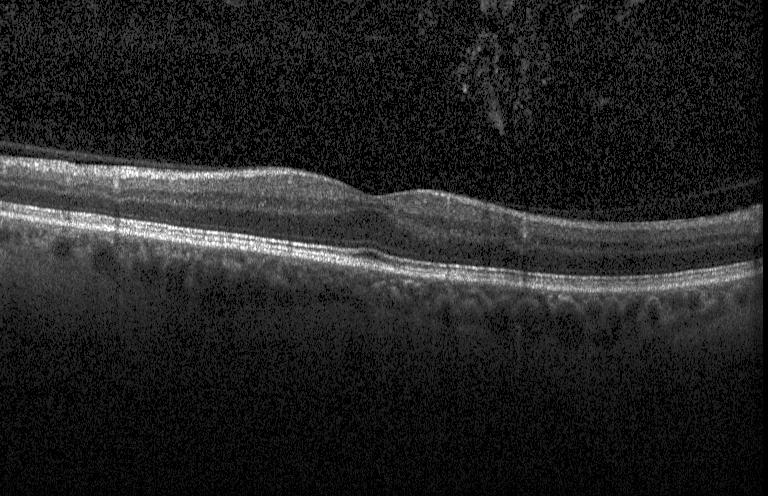

Heidelberg Spectralis OCT system; spectral-domain optical coherence tomography; OCT B-scan; macular scan — This B-scan demonstrates neither CNV, DME, nor drusen.